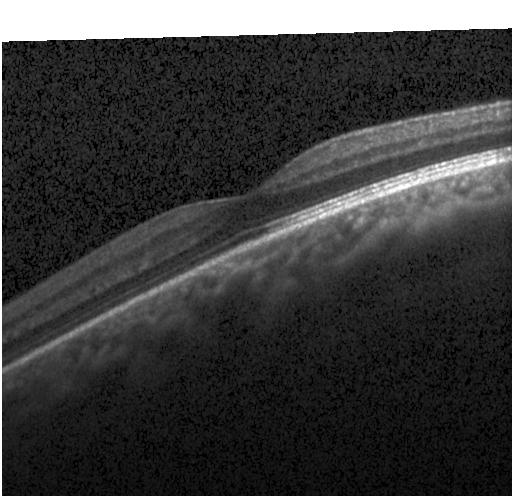

OCT finding: neither choroidal neovascularization, diabetic macular edema, nor drusen.